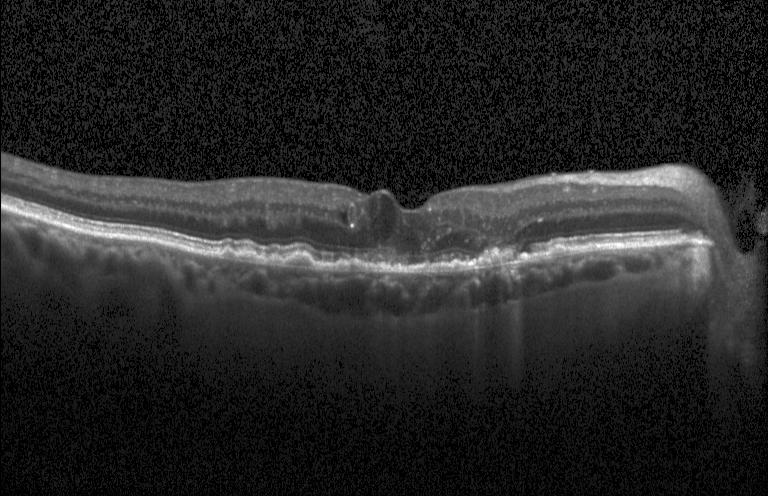 Assessment: choroidal neovascularization.